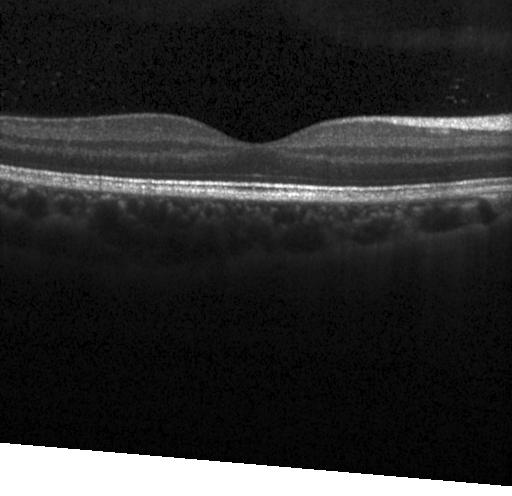 Fovea-centered, retinal OCT B-scan — OCT finding: no evidence of choroidal neovascularization, diabetic macular edema, or drusen.